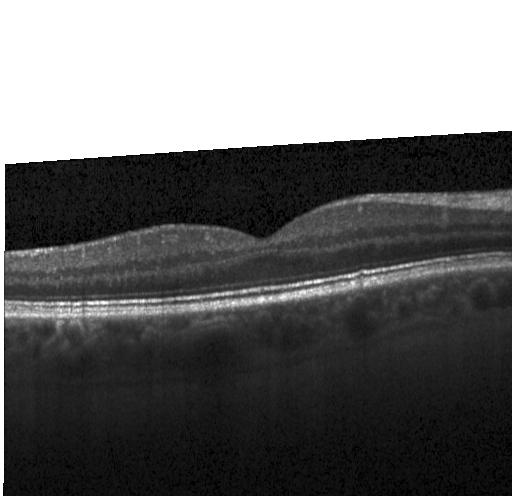

OCT scan showing no choroidal neovascularization, no diabetic macular edema, and no drusen.